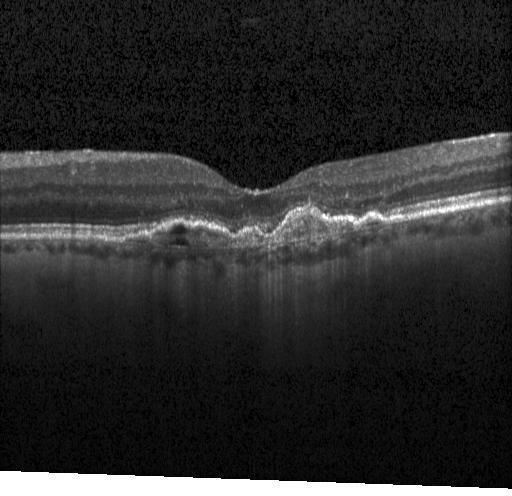 OCT B-scan · instrument: Heidelberg Spectralis · SD-OCT
Macular OCT: CNV.